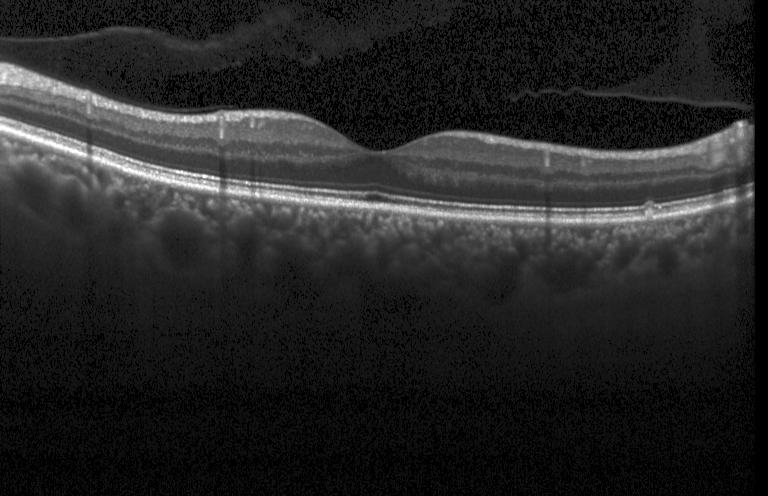 OCT line scan, centered on the fovea — Diagnosis: no choroidal neovascularization, diabetic macular edema, or drusen.